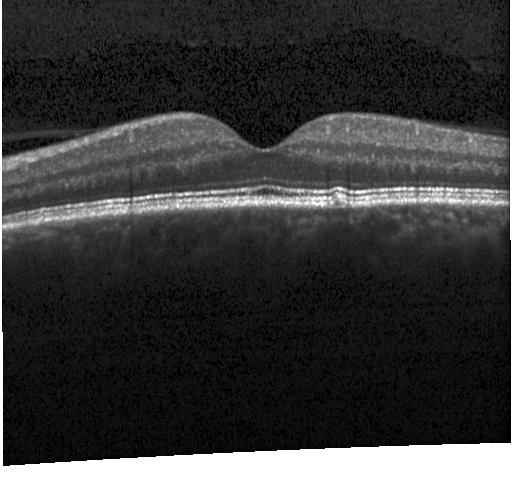
Optical coherence tomography B-scan
This B-scan demonstrates sub-RPE drusenoid deposits.